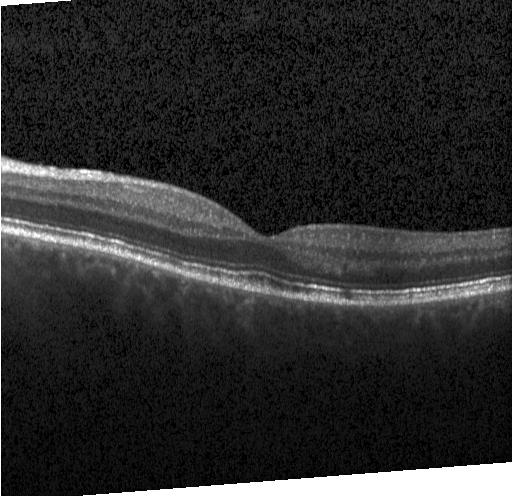 OCT B-scan
Assessment: no CNV, no DME, and no drusen.